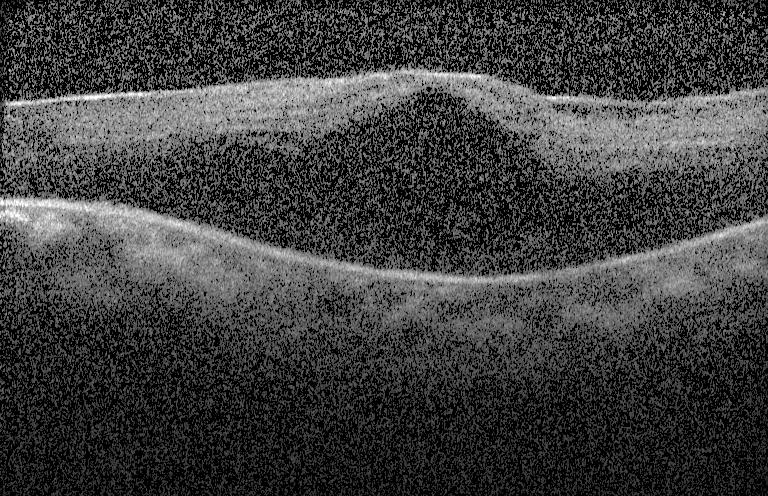
OCT line scan. Horizontal scan through the fovea
Finding: diabetic macular edema (DME).